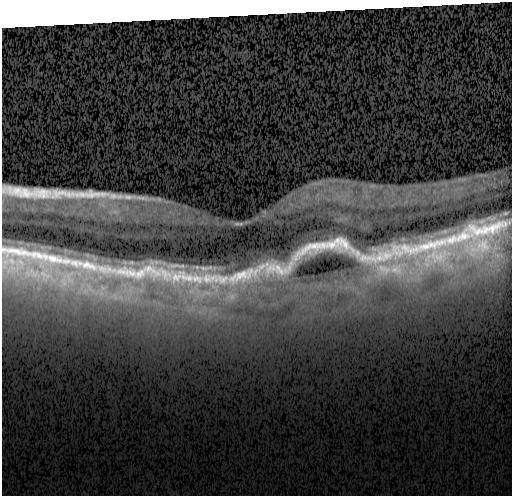

SD-OCT. Heidelberg Spectralis OCT system. Centered on the fovea. Optical coherence tomography scan. Diagnosis: a choroidal neovascular membrane.